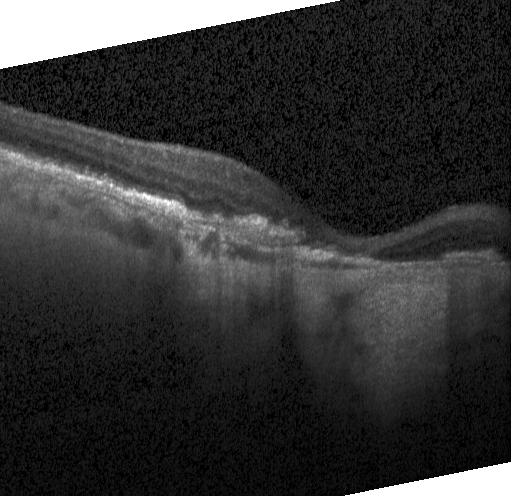

Spectral-domain optical coherence tomography, retinal OCT B-scan, acquired on a Heidelberg Spectralis, macular scan — Dx: CNV.